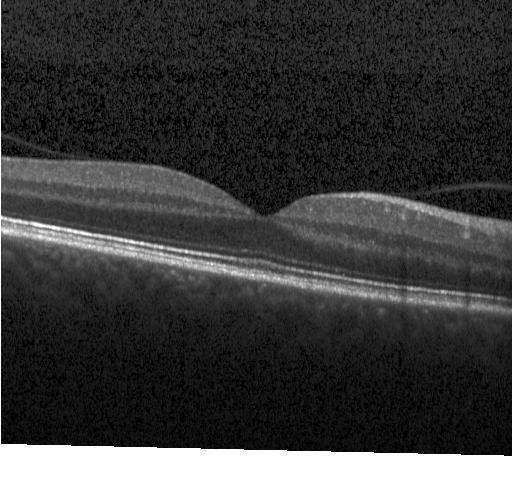 OCT finding: no evidence of choroidal neovascularization, diabetic macular edema, or drusen.